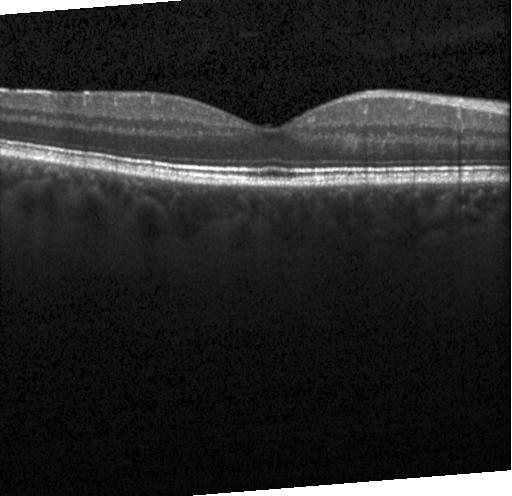 Retinal OCT B-scan. SD-OCT. Fovea-centered. Acquired on a Heidelberg Spectralis. Finding: no evidence of choroidal neovascularization, diabetic macular edema, or drusen.